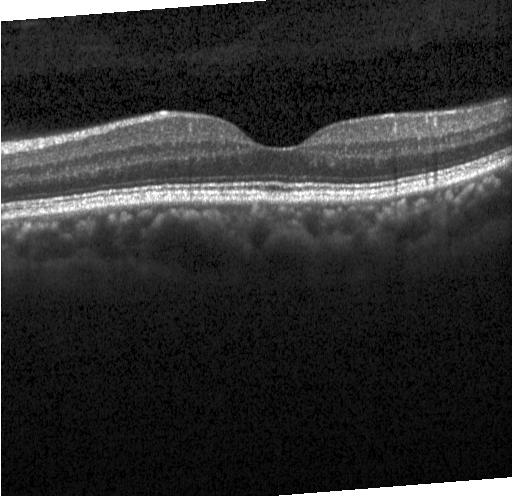
OCT finding: no choroidal neovascularization, diabetic macular edema, or drusen.